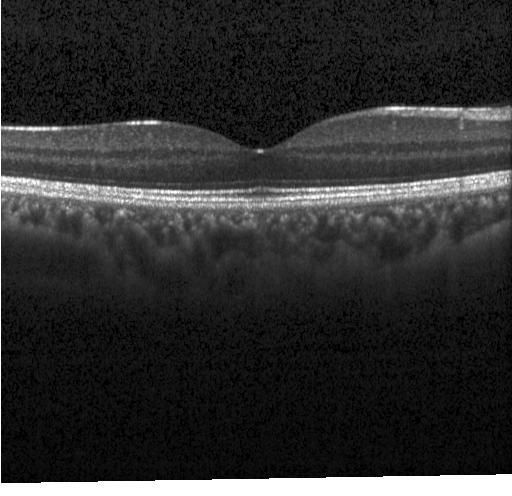 Heidelberg Spectralis, SD-OCT, optical coherence tomography scan. OCT finding: no evidence of choroidal neovascularization, diabetic macular edema, or drusen.